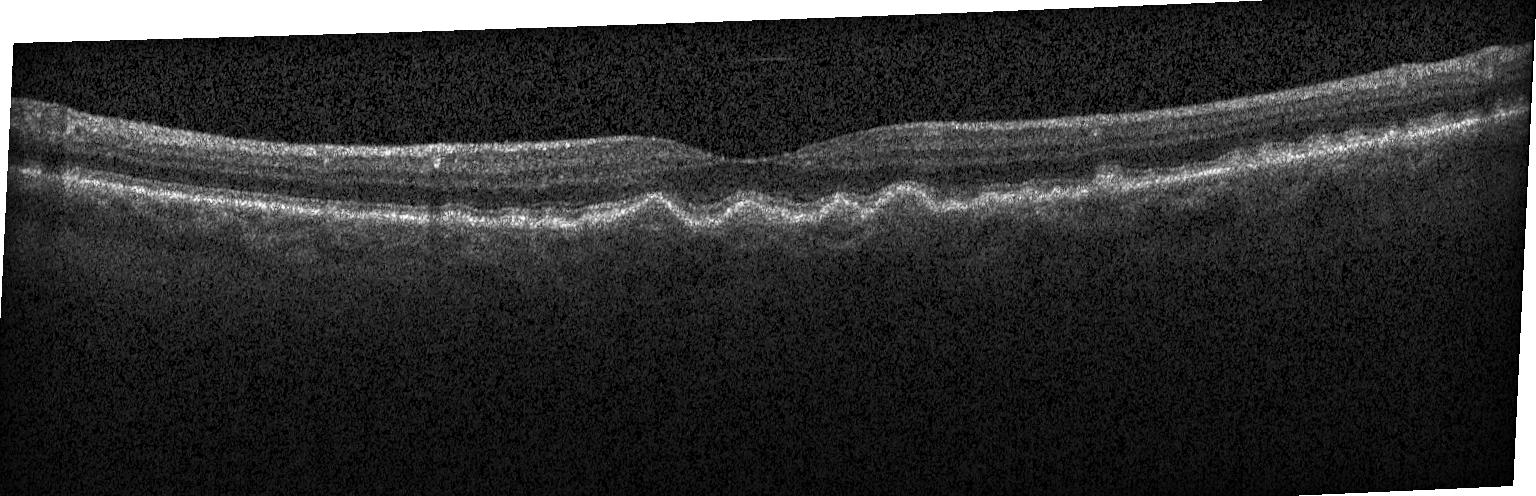 Fovea-centered, spectral-domain optical coherence tomography, retinal OCT cross-section.
Dx: drusen.